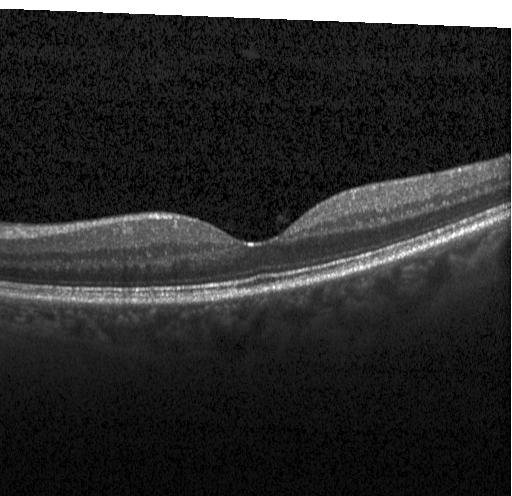
Finding: no choroidal neovascularization, no diabetic macular edema, and no drusen.